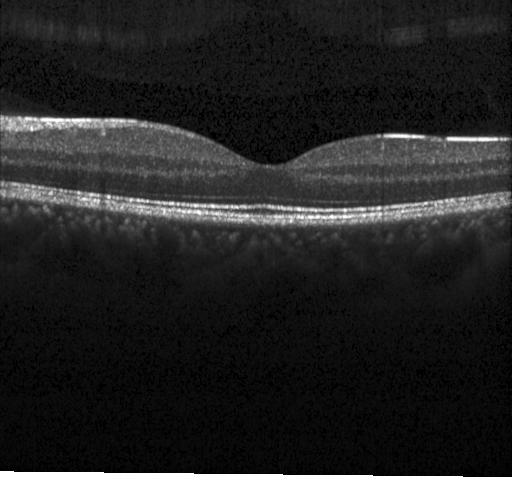 OCT line scan. Macular OCT: neither choroidal neovascularization, diabetic macular edema, nor drusen.